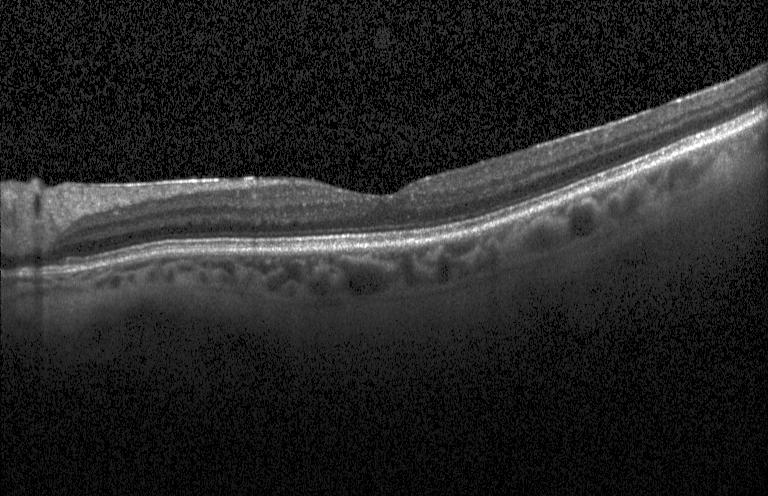

Impression: no choroidal neovascularization, no diabetic macular edema, and no drusen.